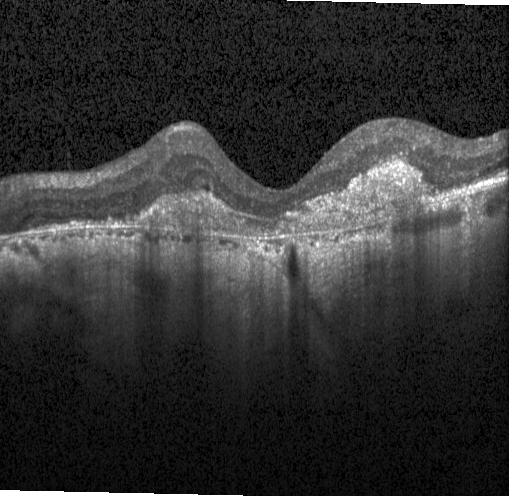

Optical coherence tomography B-scan. Impression: a choroidal neovascular membrane.